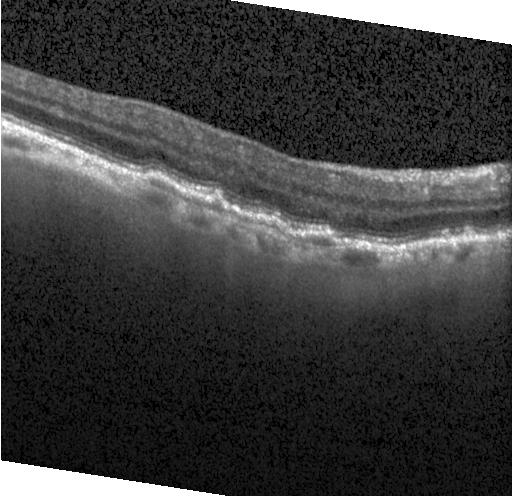 Assessment: CNV.